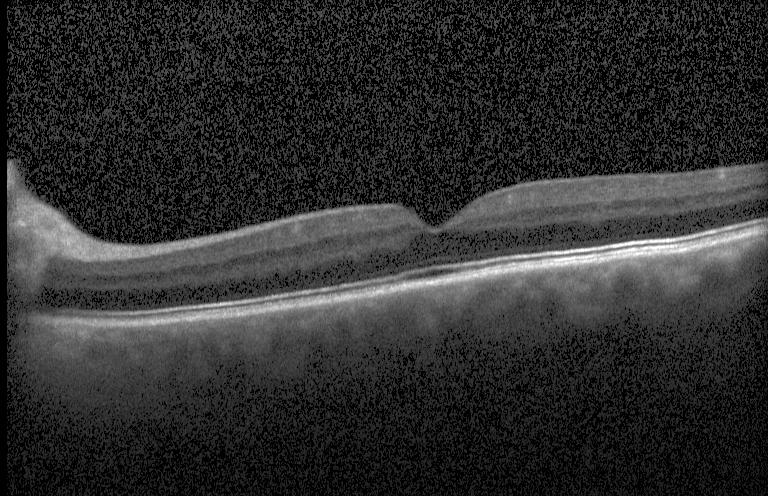
Retinal OCT cross-section showing no evidence of choroidal neovascularization, diabetic macular edema, or drusen.